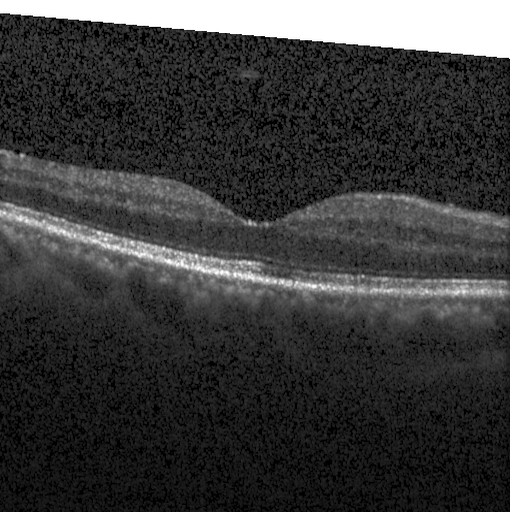

Horizontal scan through the fovea. OCT B-scan. Heidelberg Spectralis OCT system.
Diabetic macular edema.